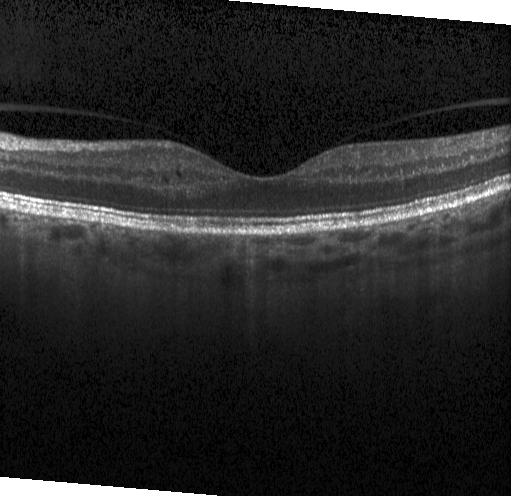

Heidelberg Spectralis; retinal OCT B-scan — Macular OCT: diabetic macular edema (DME).